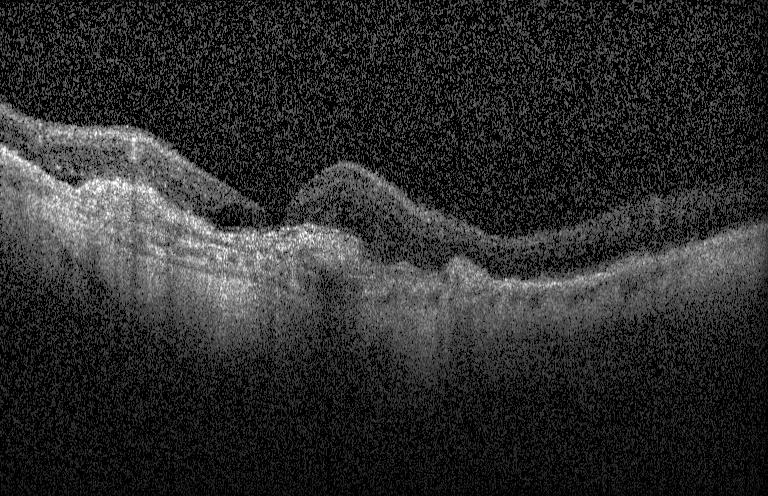 Optical coherence tomography B-scan. Spectral-domain optical coherence tomography. Instrument: Heidelberg Spectralis. Macular OCT: choroidal neovascularization (CNV).